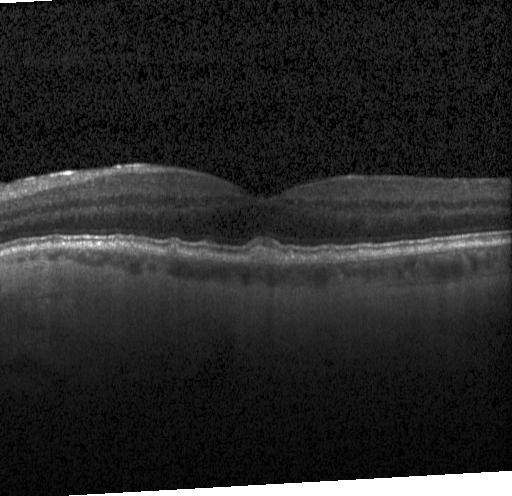 Dx: multiple drusen.